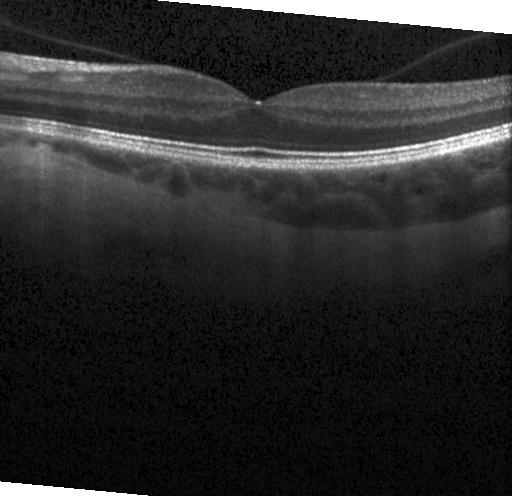

OCT B-scan showing no evidence of choroidal neovascularization, diabetic macular edema, or drusen.